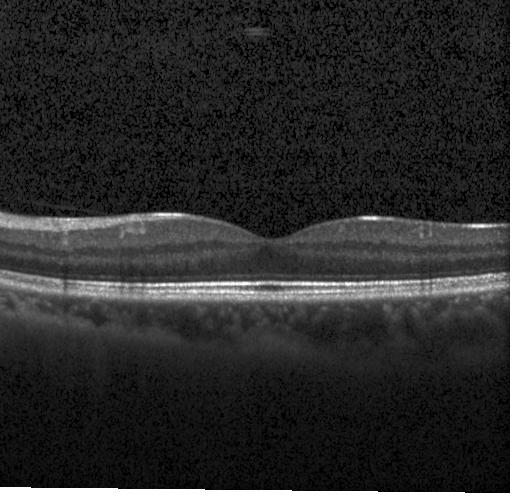
Horizontal scan through the fovea, retinal OCT B-scan. This B-scan demonstrates no choroidal neovascularization, diabetic macular edema, or drusen.